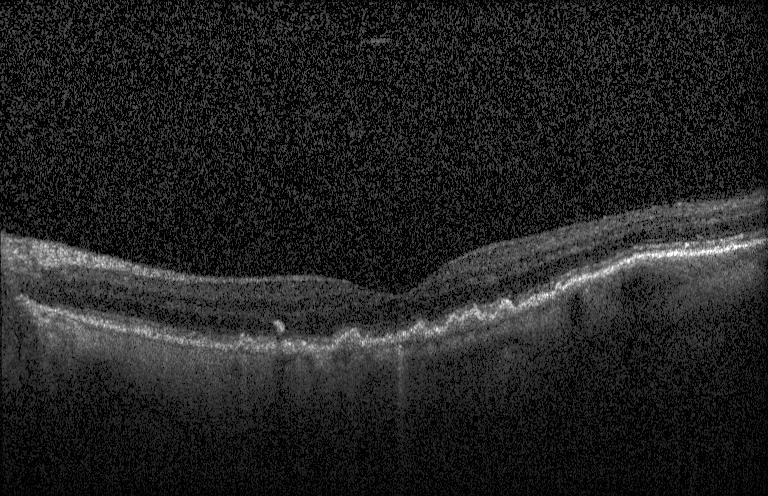

Assessment: multiple drusen.